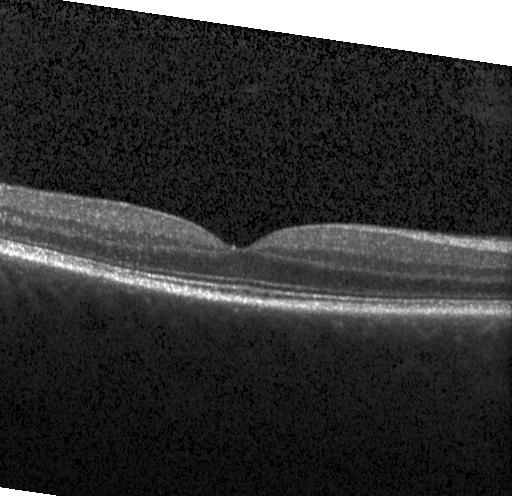
OCT line scan, through the macula, instrument: Heidelberg Spectralis — Macular OCT: no CNV, no DME, and no drusen.